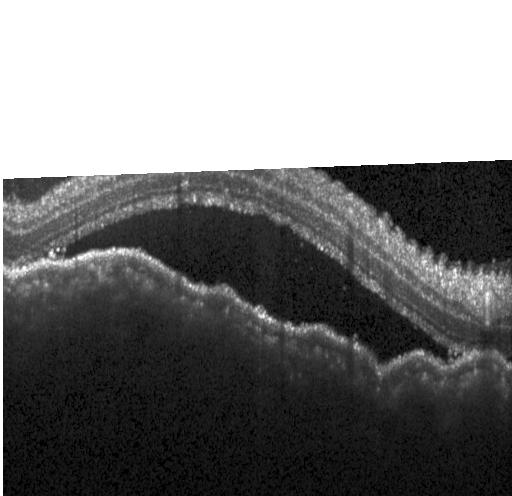
OCT B-scan showing choroidal neovascularization.